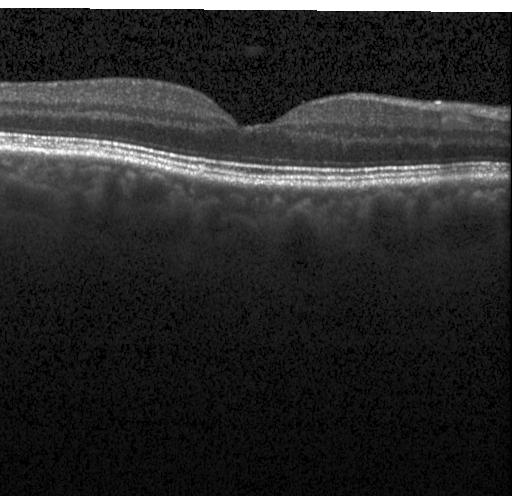

Dx: no CNV, DME, or drusen.